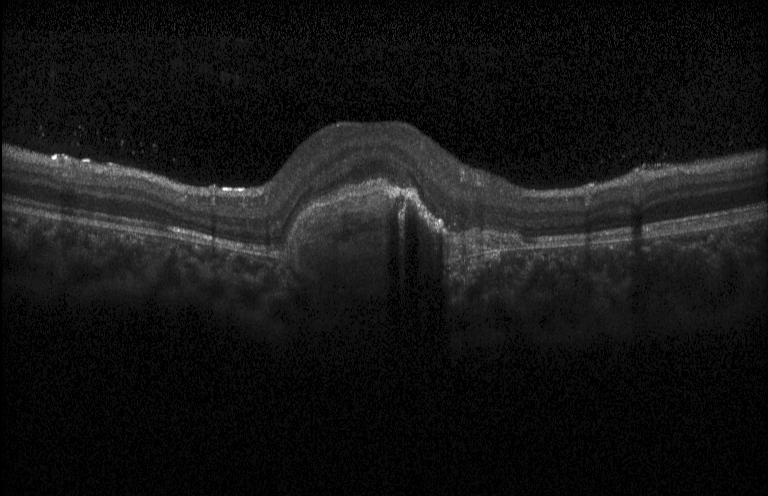
Spectral-domain OCT. OCT B-scan
Diagnosis: a choroidal neovascular membrane.